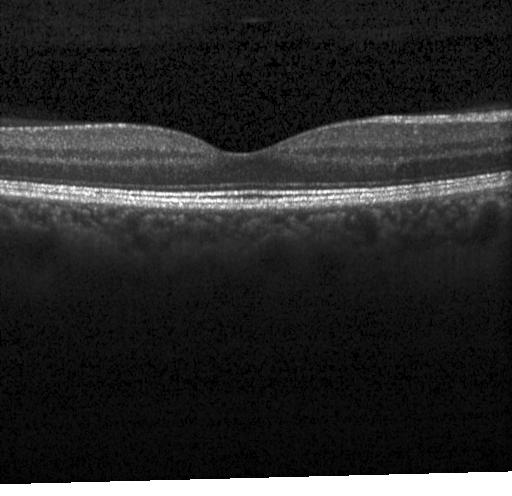 SD-OCT; instrument: Heidelberg Spectralis; macular scan; optical coherence tomography scan.
Finding: no choroidal neovascularization, no diabetic macular edema, and no drusen.